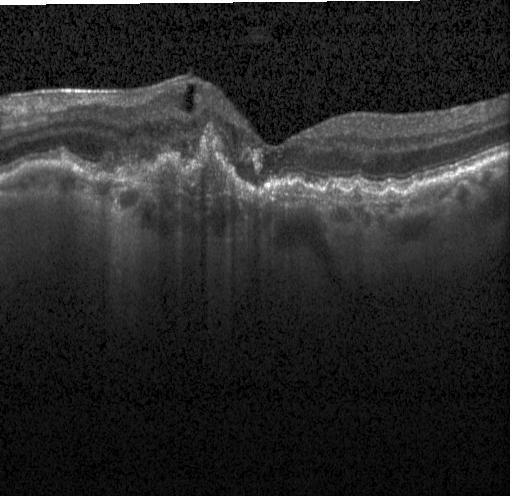 Acquired on a Heidelberg Spectralis; SD-OCT; optical coherence tomography B-scan. Dx: a choroidal neovascular membrane.